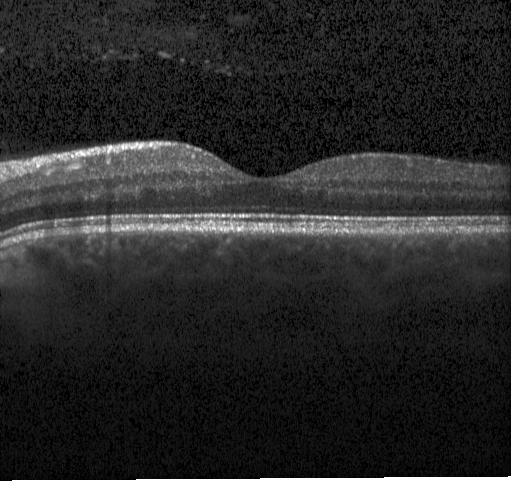

Optical coherence tomography B-scan, horizontal scan through the fovea
No evidence of choroidal neovascularization, diabetic macular edema, or drusen.